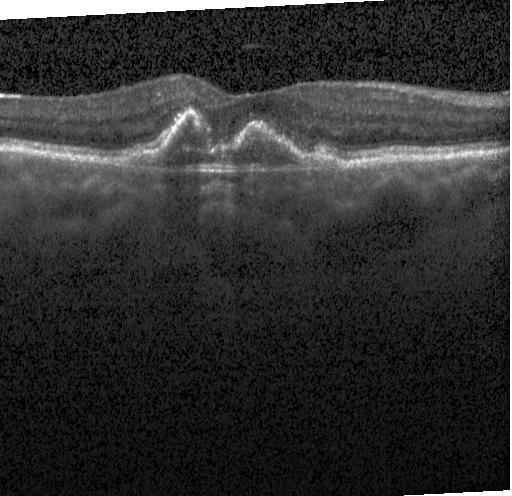
OCT line scan.
Finding: a choroidal neovascular membrane.